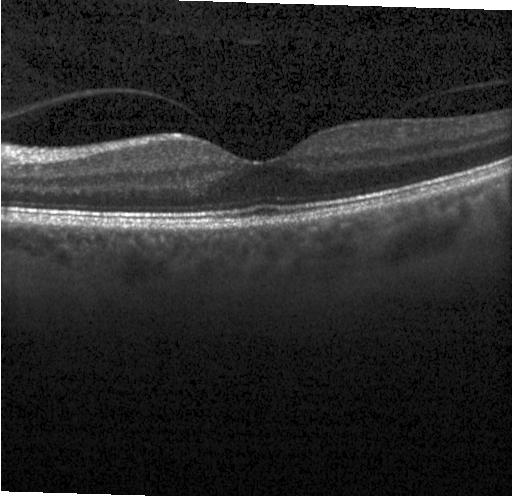 OCT scan showing no CNV, DME, or drusen.